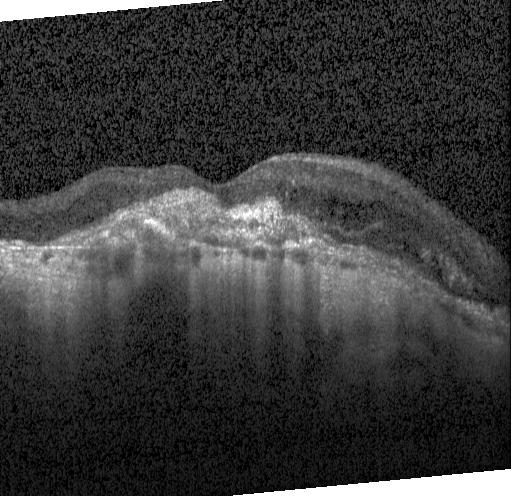

SD-OCT · OCT line scan · centered on the fovea · instrument: Heidelberg Spectralis.
Impression: a choroidal neovascular membrane.